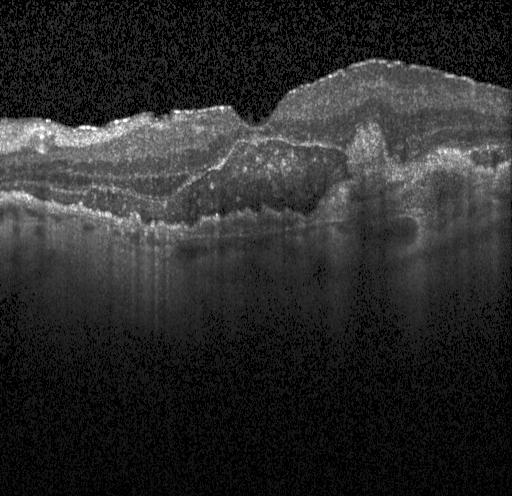
Spectral-domain OCT · horizontal scan through the fovea · instrument: Heidelberg Spectralis · retinal OCT B-scan
Finding: a choroidal neovascular membrane.